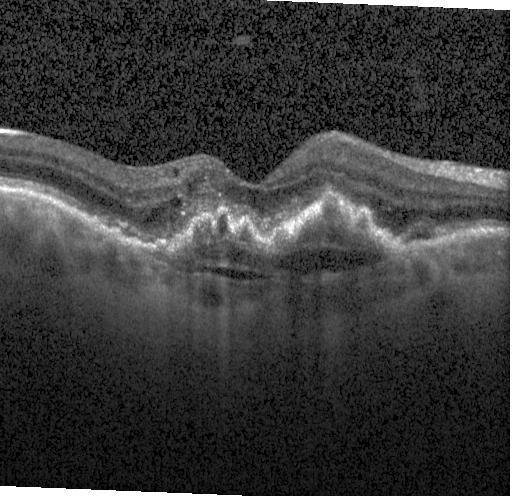
Diagnosis: choroidal neovascularization.